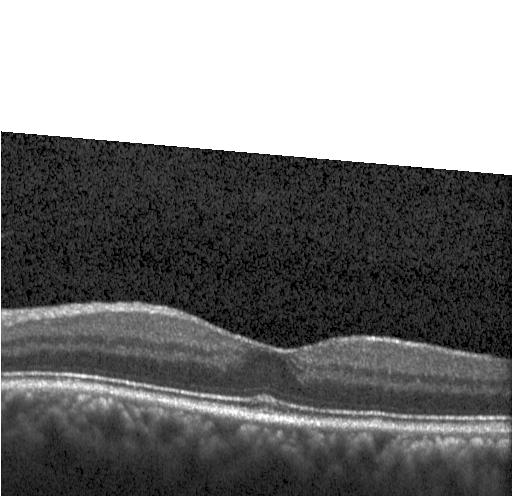 Optical coherence tomography scan. Macular scan. Impression: no evidence of CNV, DME, or drusen.